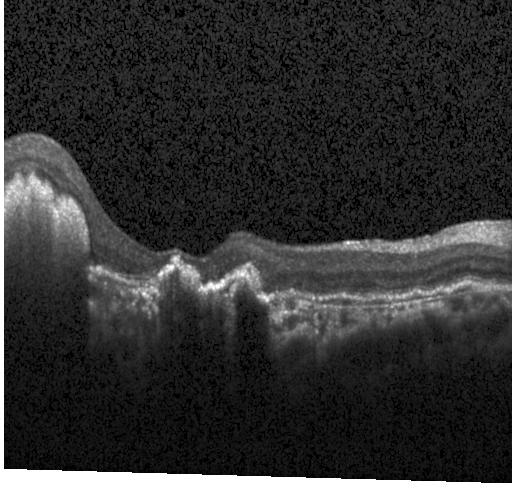 Horizontal scan through the fovea · SD-OCT · Heidelberg Spectralis · OCT B-scan.
Impression: a choroidal neovascular membrane.